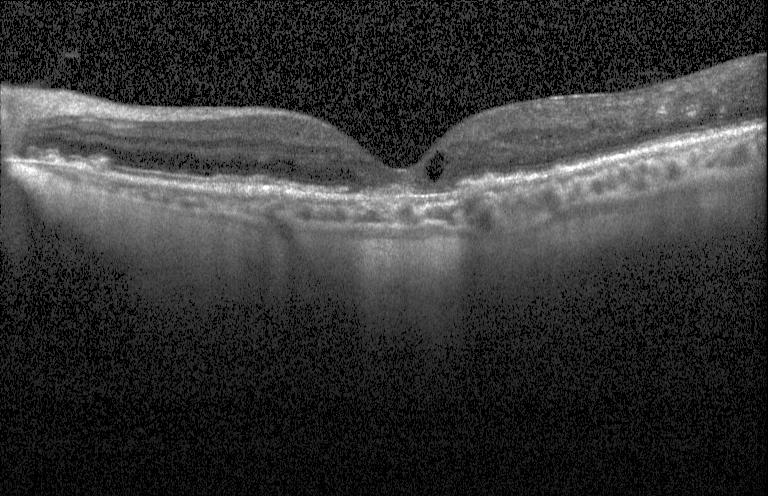

Instrument: Heidelberg Spectralis; spectral-domain optical coherence tomography; retinal OCT B-scan
Diagnosis: choroidal neovascularization.